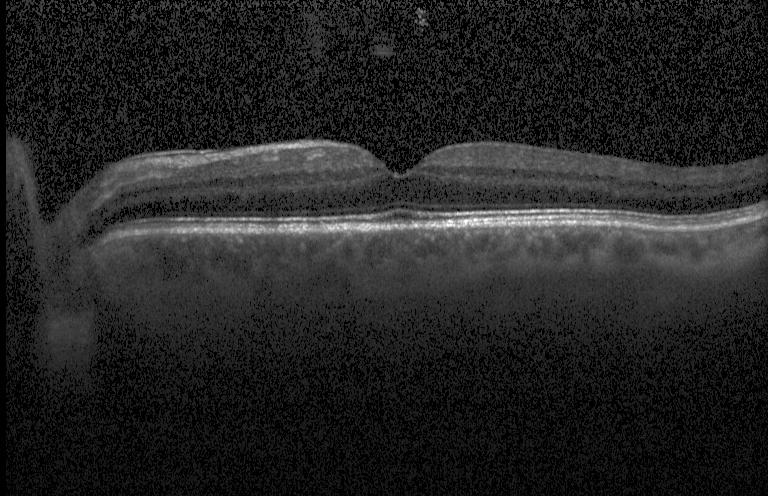 Optical coherence tomography B-scan, SD-OCT, Heidelberg Spectralis OCT system, through the macula — The scan shows neither choroidal neovascularization, diabetic macular edema, nor drusen.